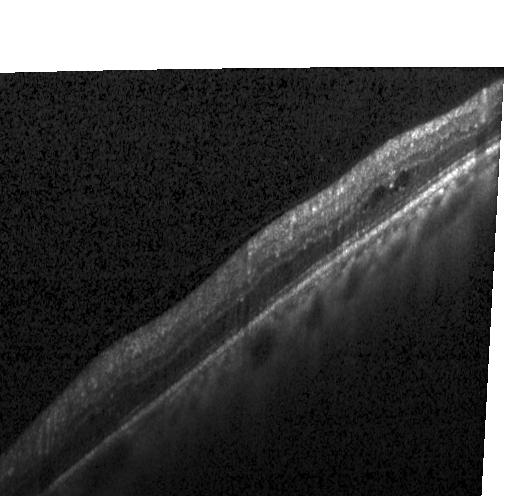

Centered on the fovea · SD-OCT · OCT B-scan
Finding: DME.